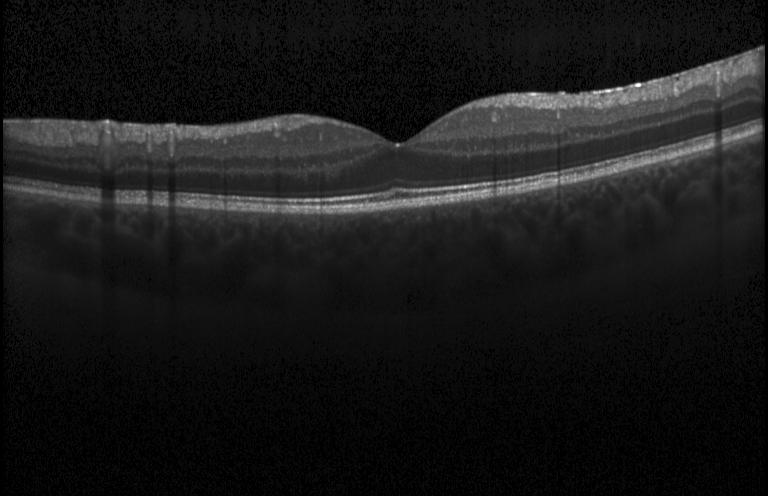 Retinal OCT B-scan · Heidelberg Spectralis OCT system. This B-scan demonstrates no CNV, DME, or drusen.